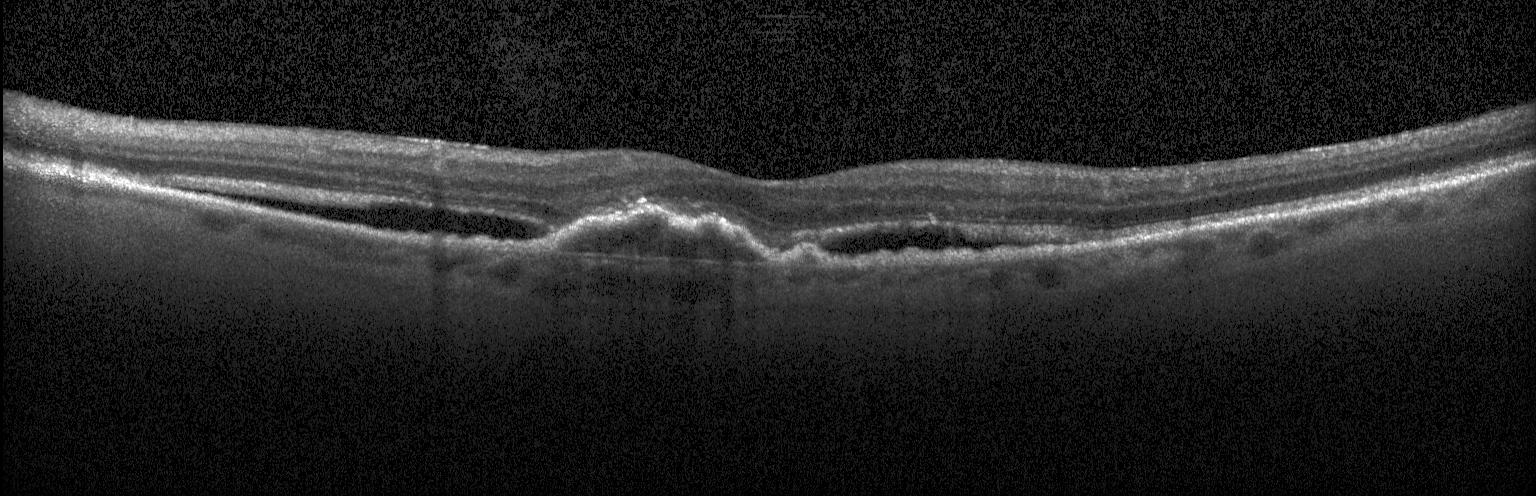
Diagnosis: a choroidal neovascular membrane.